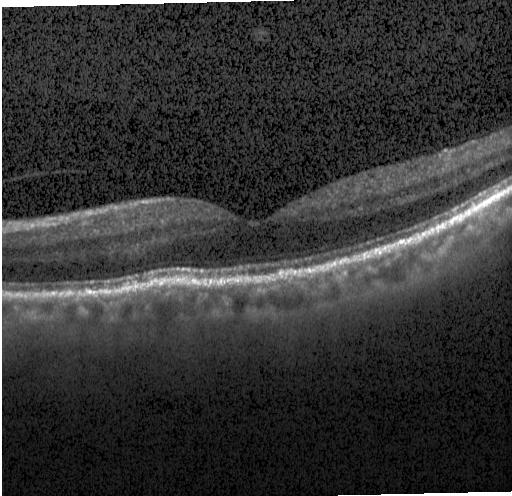
No CNV, DME, or drusen.